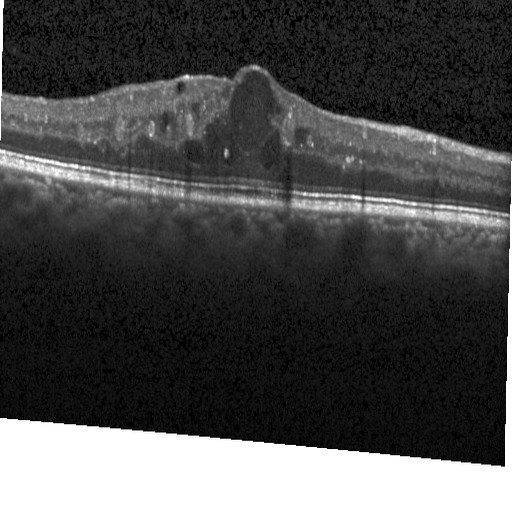 Fovea-centered, OCT line scan, spectral-domain OCT, acquired on a Heidelberg Spectralis
Macular OCT: DME.